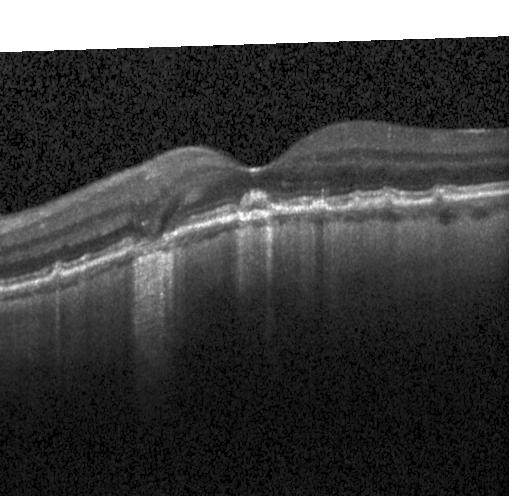
Heidelberg Spectralis, retinal OCT cross-section. Dx: choroidal neovascularization (CNV).